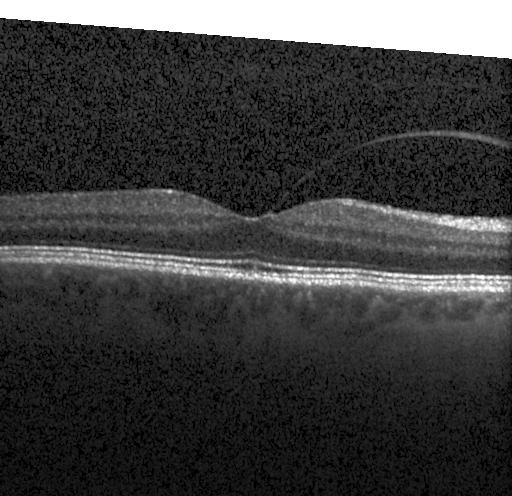
Instrument: Heidelberg Spectralis, retinal OCT B-scan, spectral-domain OCT, fovea-centered. Dx: no CNV, DME, or drusen.